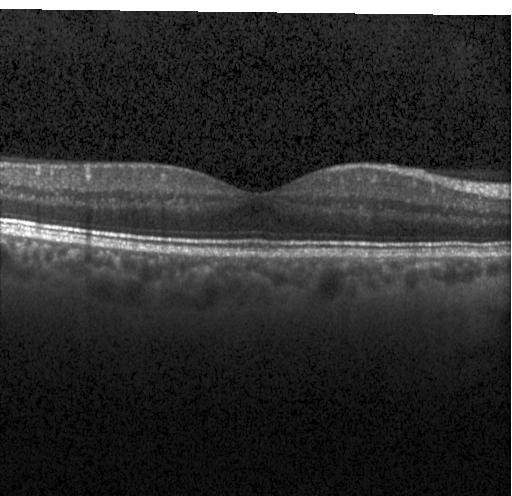

Finding: no choroidal neovascularization, diabetic macular edema, or drusen.